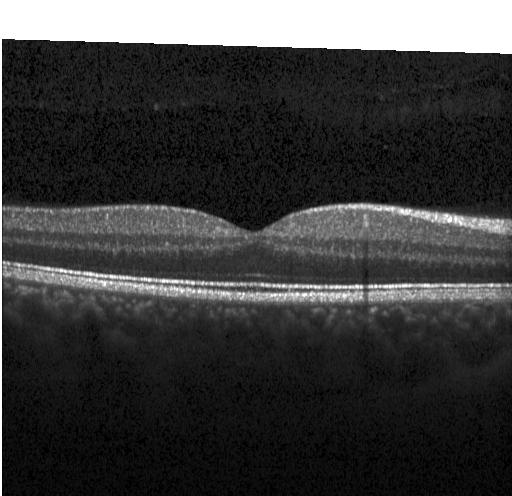
Impression: no evidence of choroidal neovascularization, diabetic macular edema, or drusen.